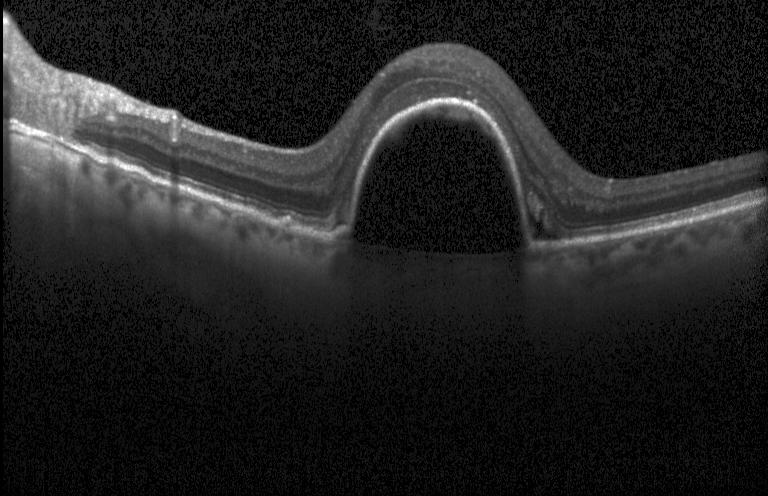
Spectral-domain OCT B-scan: a choroidal neovascular membrane.